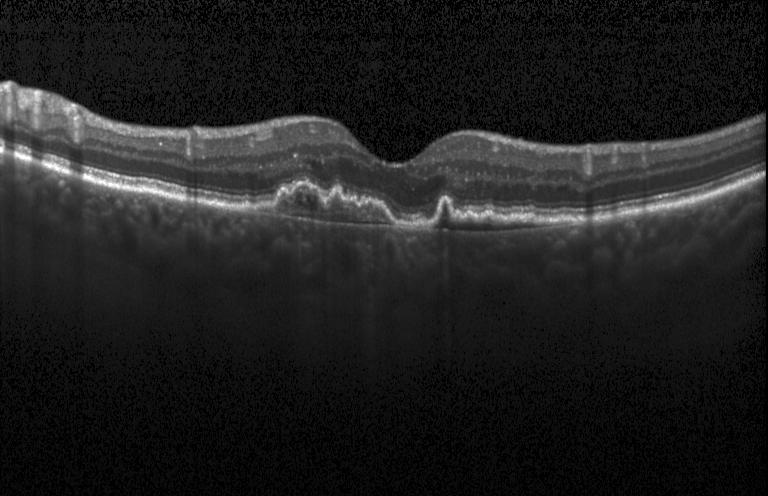
The scan shows a choroidal neovascular membrane.